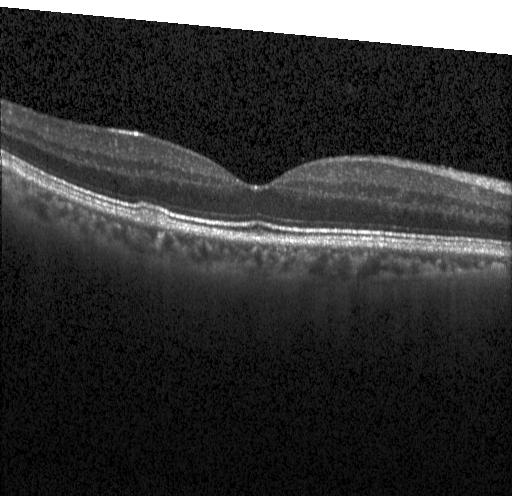 Spectral-domain optical coherence tomography; macular scan; acquired on a Heidelberg Spectralis; retinal OCT cross-section.
Drusen.